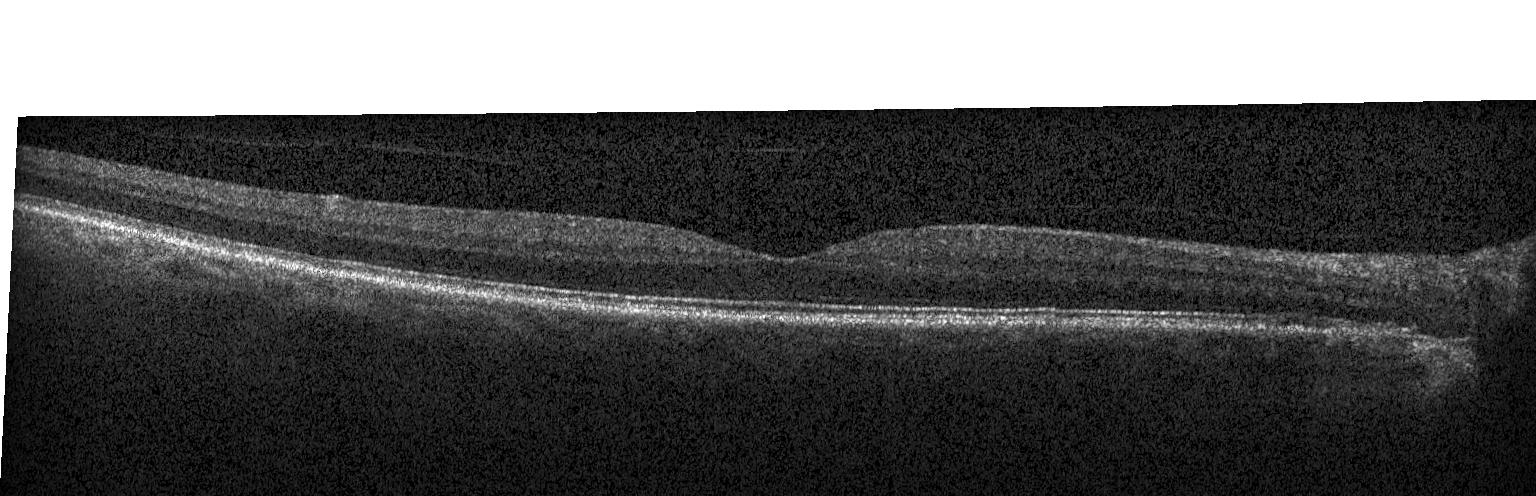
Finding: no choroidal neovascularization, no diabetic macular edema, and no drusen.